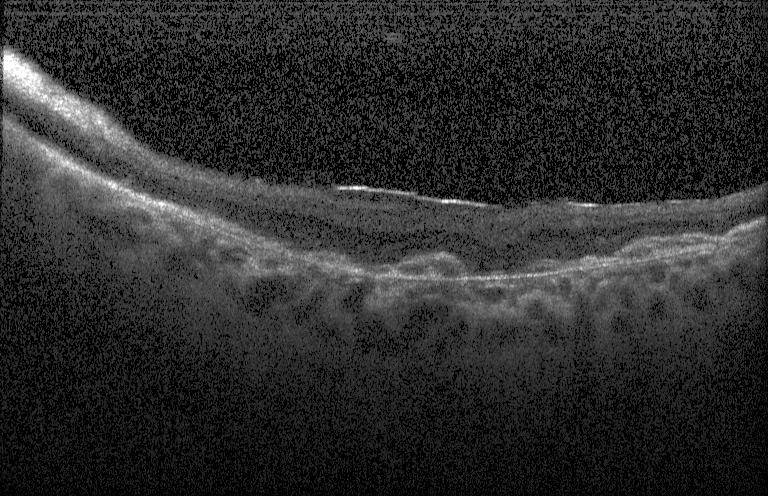 OCT line scan · spectral-domain optical coherence tomography — Finding: a choroidal neovascular membrane.